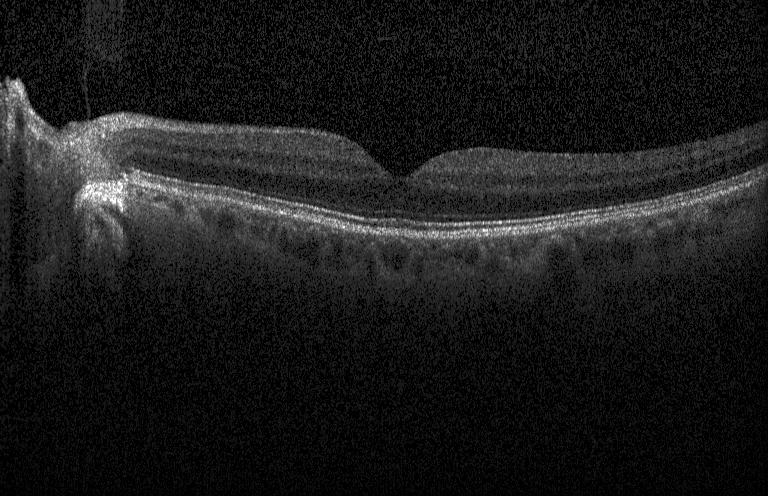
Optical coherence tomography scan. Horizontal scan through the fovea. Heidelberg Spectralis OCT system. Spectral-domain optical coherence tomography
Impression: neither CNV, DME, nor drusen.